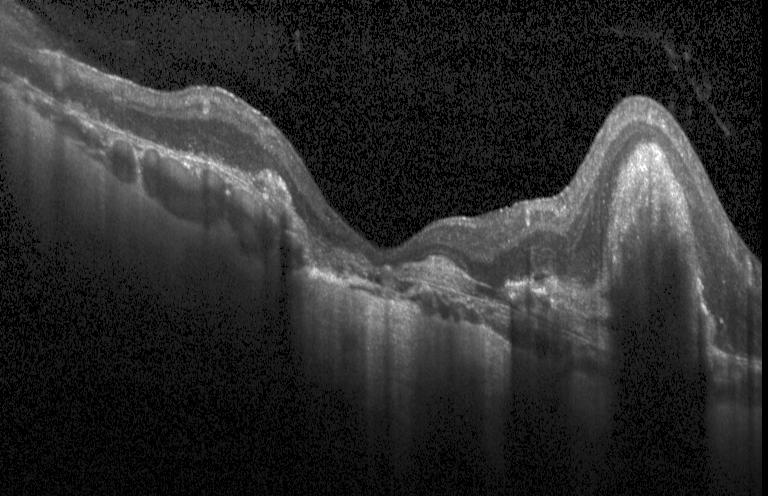 Retinal OCT cross-section showing a choroidal neovascular membrane.